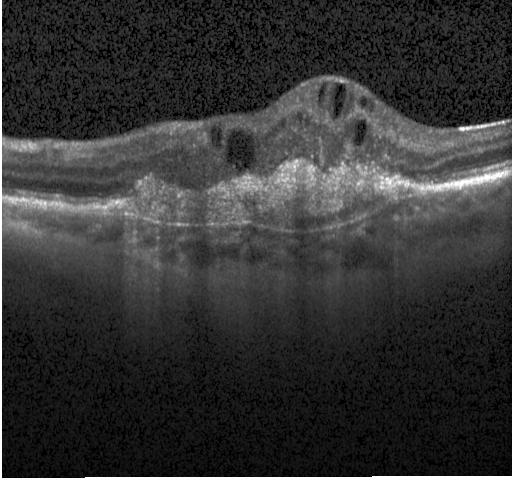
Assessment: a choroidal neovascular membrane.